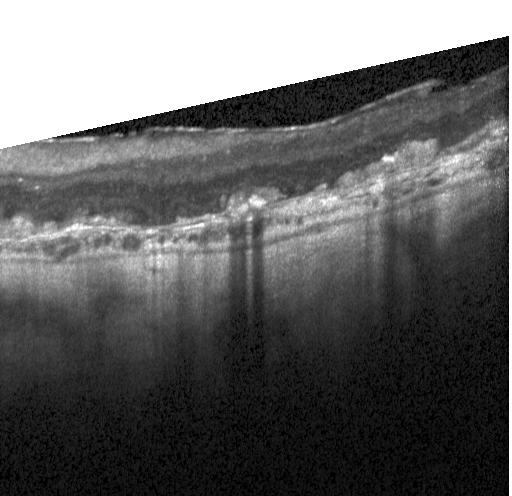 Optical coherence tomography scan; centered on the fovea
This B-scan demonstrates choroidal neovascularization (CNV).